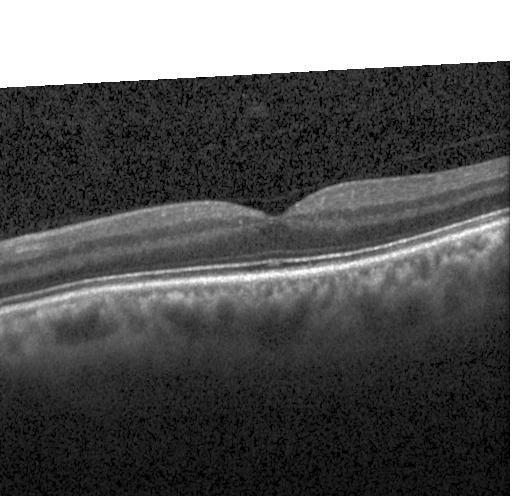
OCT finding: no evidence of CNV, DME, or drusen.